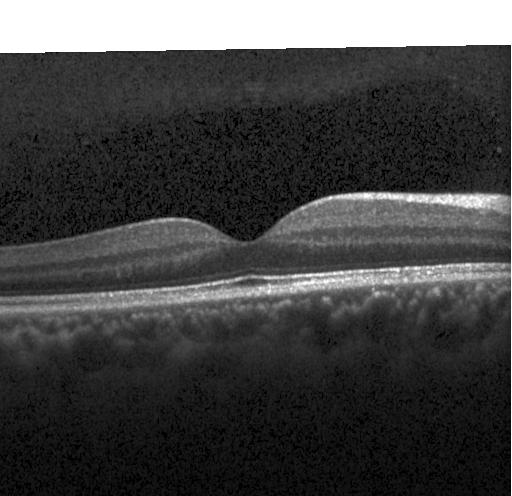 OCT scan showing no evidence of CNV, DME, or drusen.